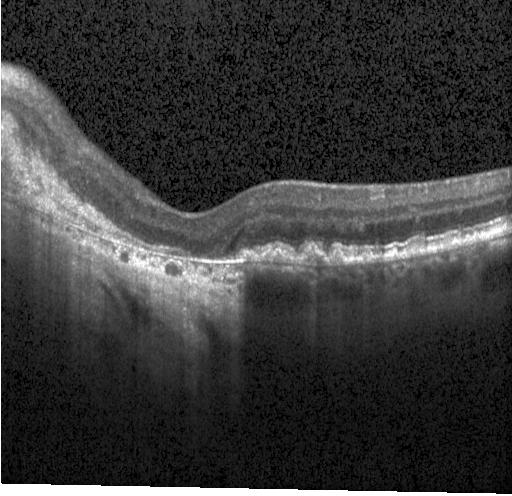

OCT finding: CNV.